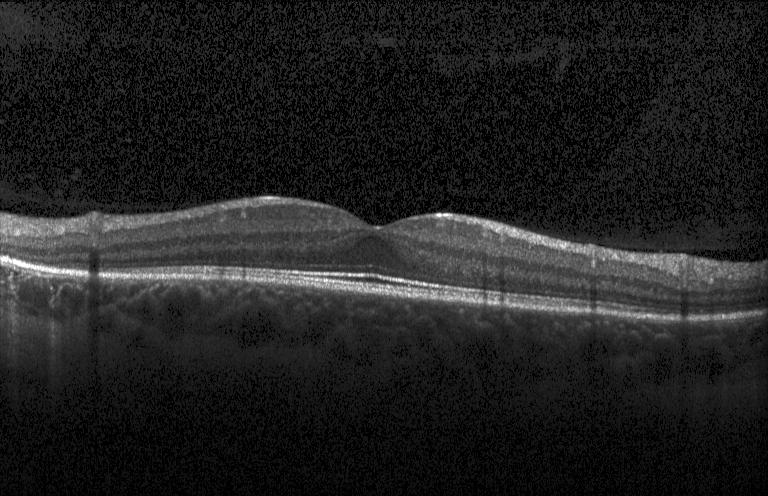
This B-scan demonstrates no evidence of CNV, DME, or drusen.